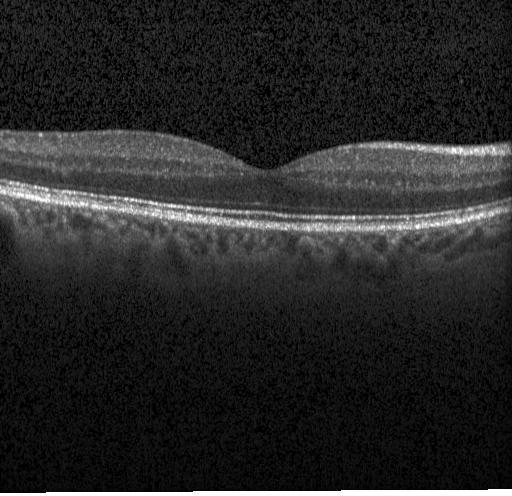
Heidelberg Spectralis. Horizontal scan through the fovea. Spectral-domain OCT. Retinal OCT B-scan.
Dx: neither CNV, DME, nor drusen.